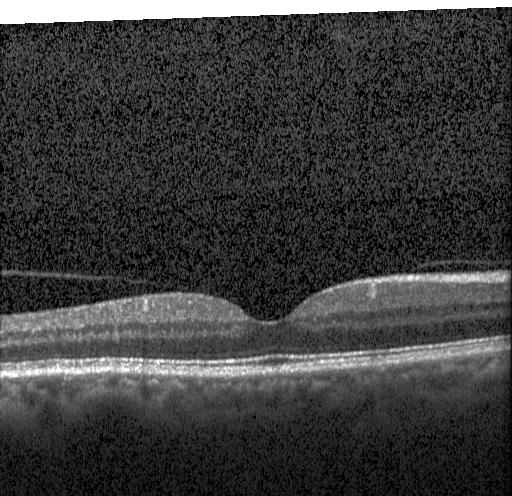

SD-OCT; optical coherence tomography scan.
Diagnosis: no choroidal neovascularization, diabetic macular edema, or drusen.